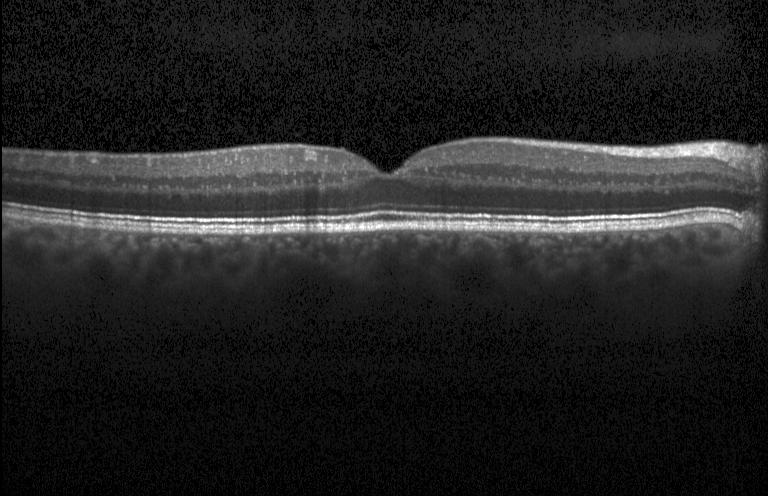 No CNV, DME, or drusen.